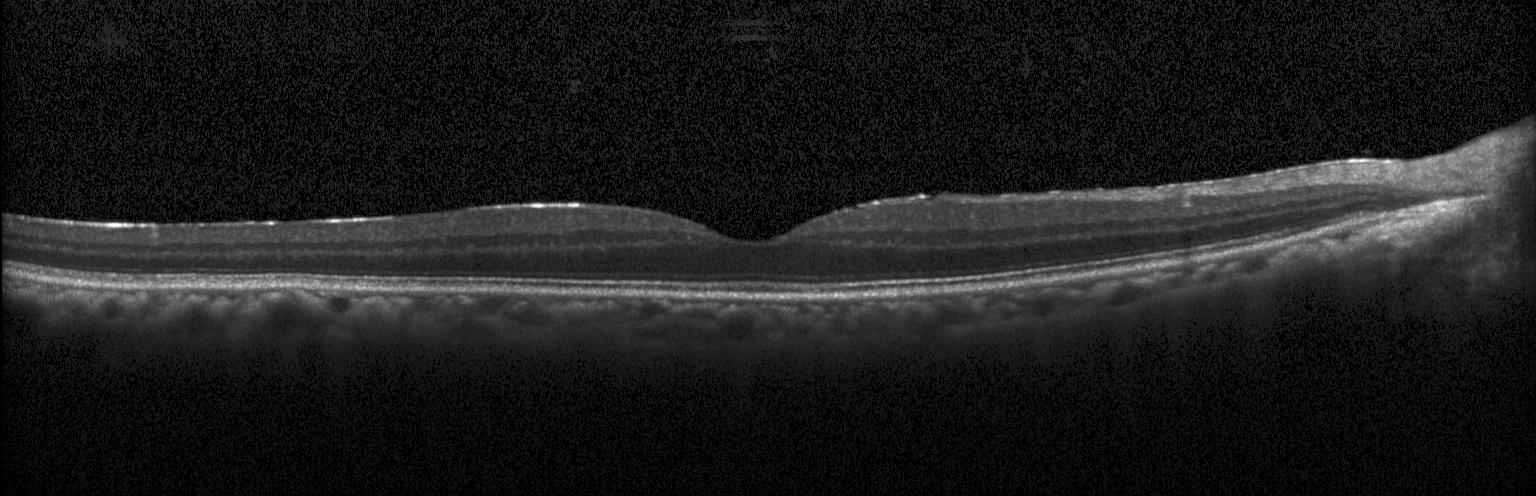
This B-scan demonstrates neither CNV, DME, nor drusen.